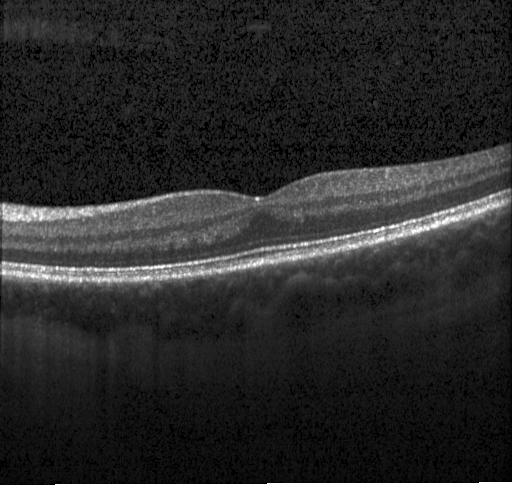 The scan shows no evidence of choroidal neovascularization, diabetic macular edema, or drusen.